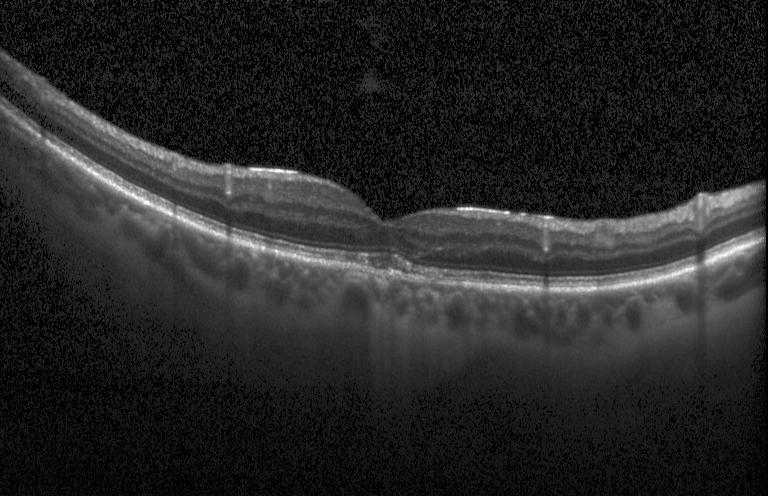
OCT B-scan · spectral-domain OCT · through the macula. Dx: choroidal neovascularization (CNV).